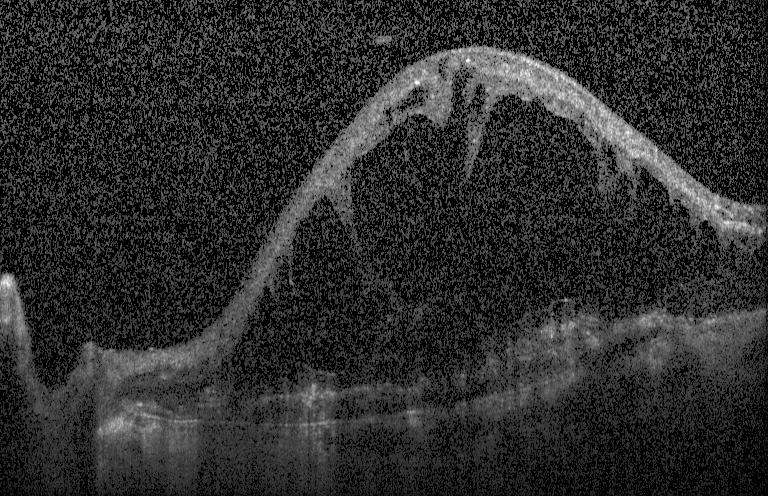 Impression: CNV.